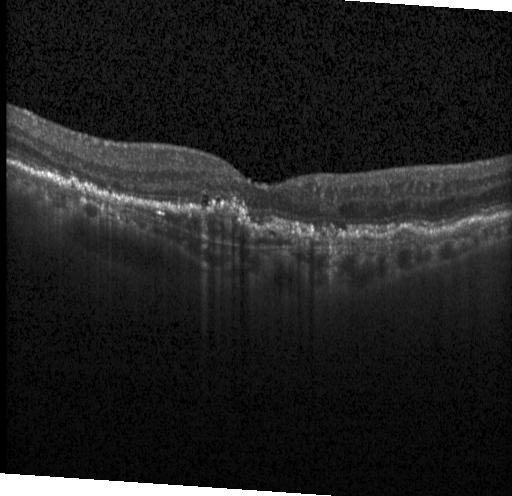 Optical coherence tomography B-scan. Impression: choroidal neovascularization.